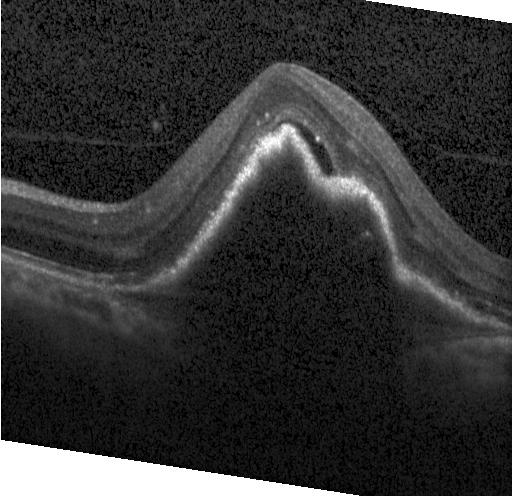
Spectral-domain OCT B-scan: CNV.